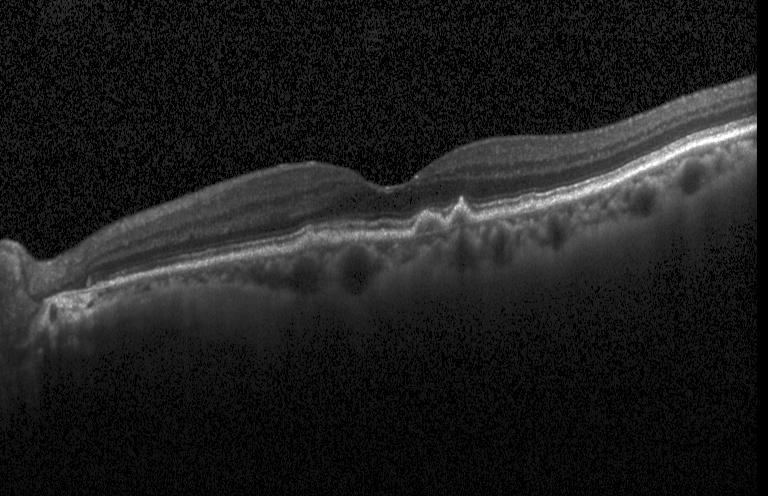
Impression: drusen.